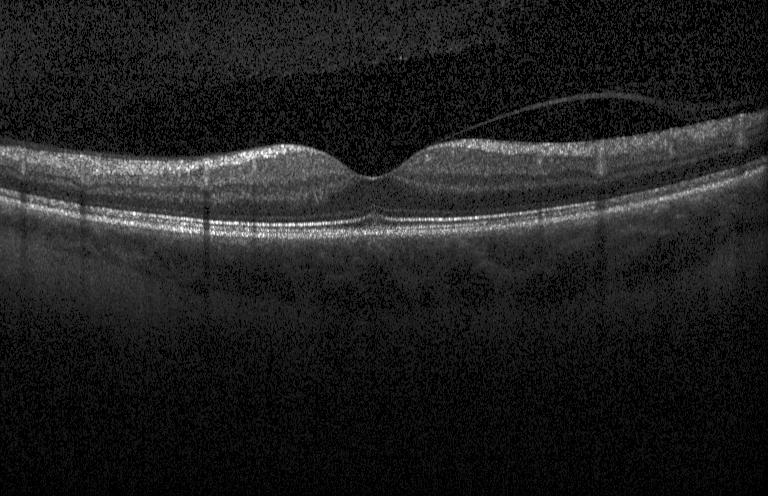

Optical coherence tomography scan, Heidelberg Spectralis
OCT finding: no evidence of choroidal neovascularization, diabetic macular edema, or drusen.